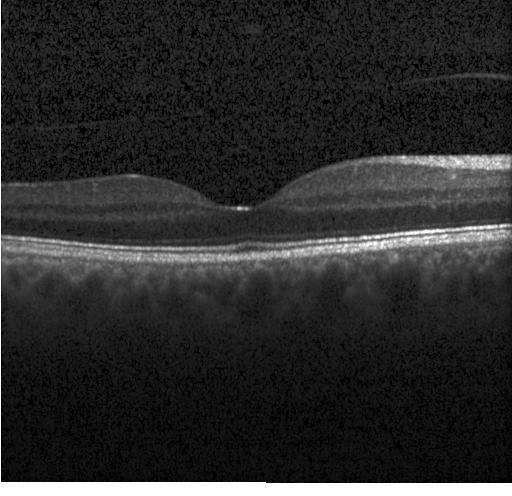 Impression: no choroidal neovascularization, diabetic macular edema, or drusen.